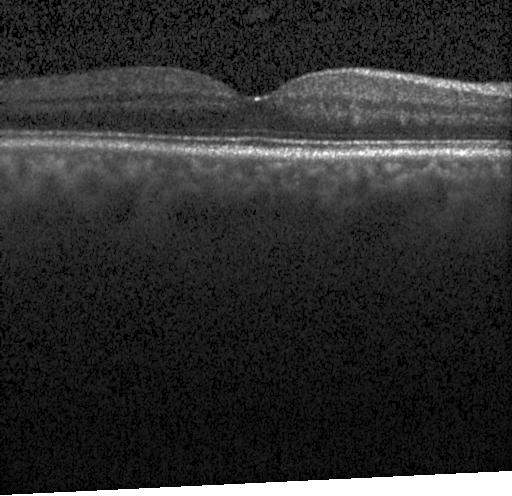

Optical coherence tomography B-scan · instrument: Heidelberg Spectralis — Macular OCT: neither CNV, DME, nor drusen.